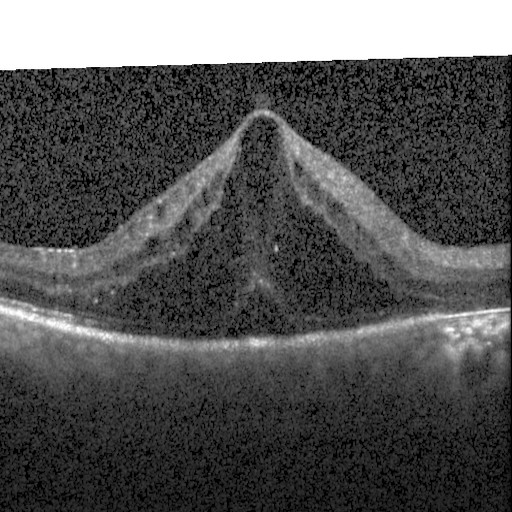 Macular OCT demonstrating diabetic macular edema.